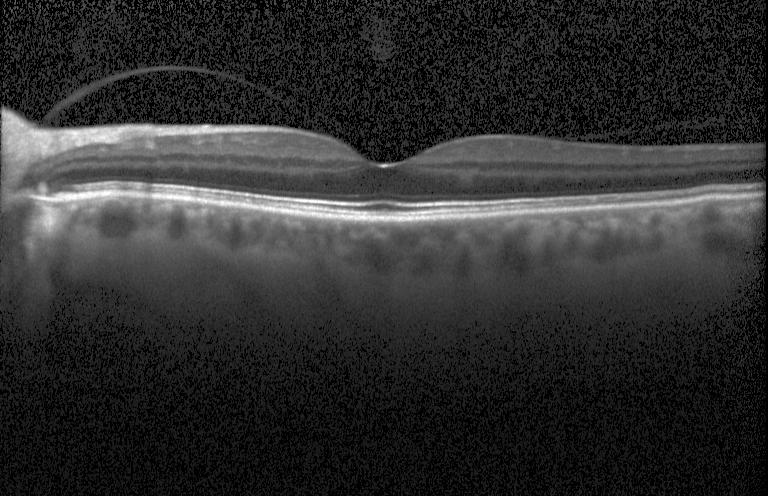
OCT scan showing no CNV, no DME, and no drusen.